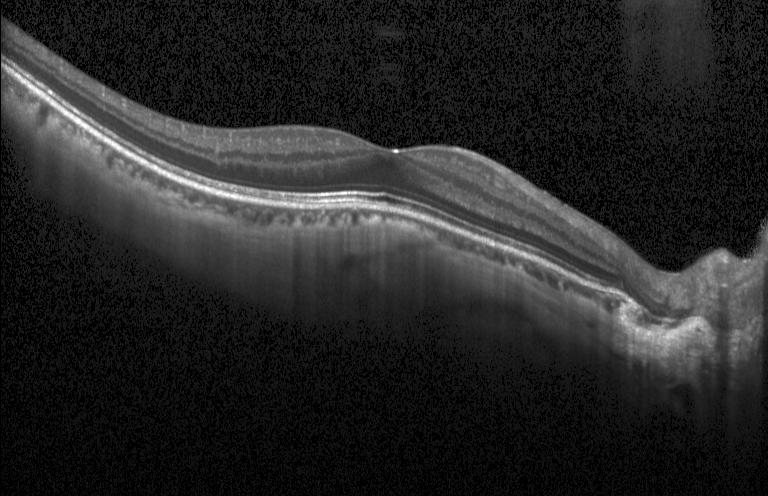 Acquired on a Heidelberg Spectralis, spectral-domain OCT, OCT B-scan, through the macula — Impression: no choroidal neovascularization, diabetic macular edema, or drusen.